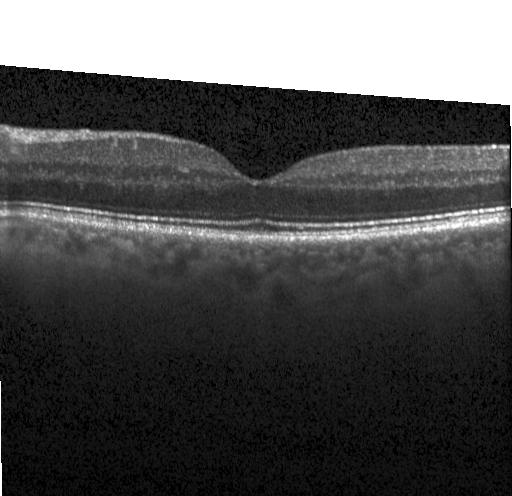

OCT line scan, spectral-domain optical coherence tomography.
Finding: no choroidal neovascularization, no diabetic macular edema, and no drusen.